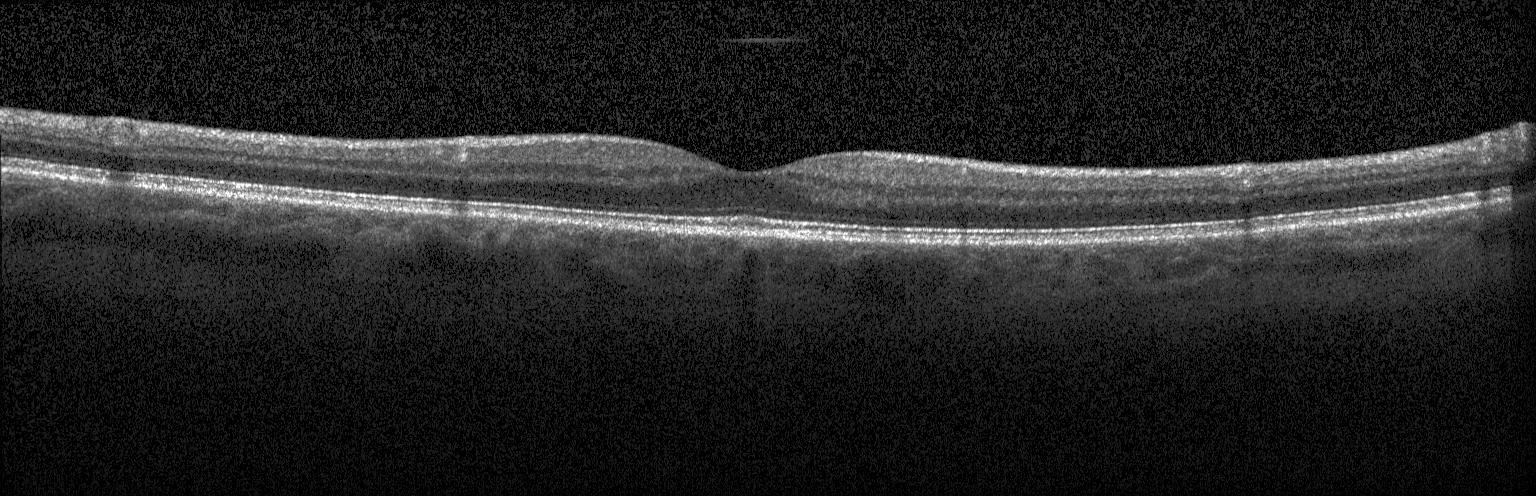
OCT line scan — No evidence of choroidal neovascularization, diabetic macular edema, or drusen.